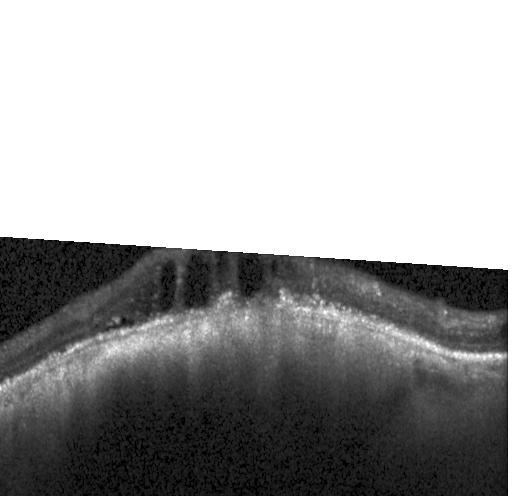
Spectral-domain OCT B-scan: choroidal neovascularization.